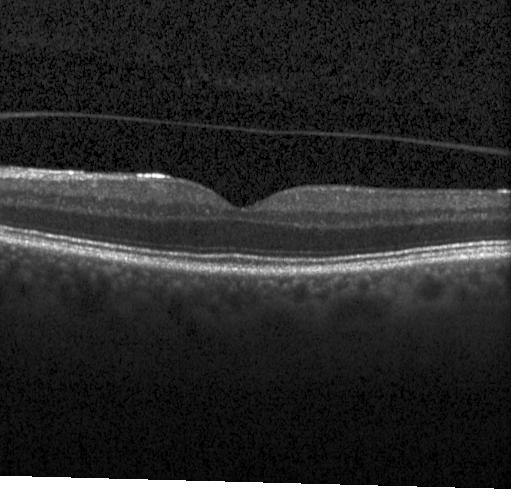
OCT B-scan, horizontal scan through the fovea.
This B-scan demonstrates no choroidal neovascularization, no diabetic macular edema, and no drusen.